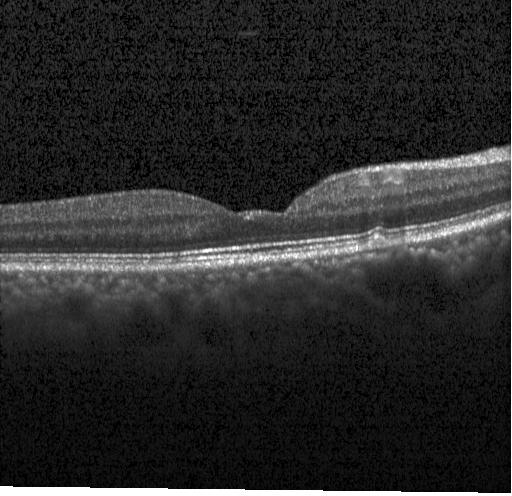
Spectral-domain OCT. Horizontal scan through the fovea. Retinal OCT B-scan. Heidelberg Spectralis OCT system — Diagnosis: multiple drusen.